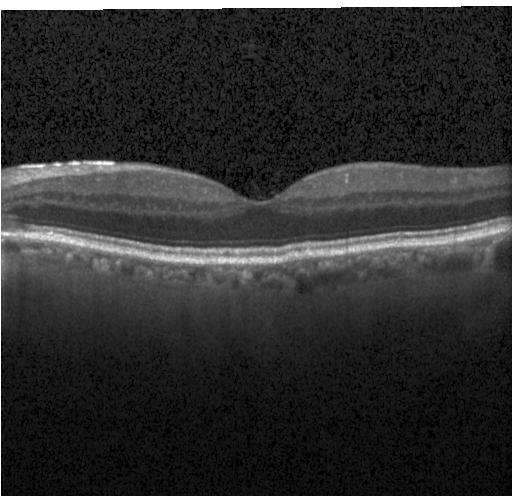

Retinal OCT B-scan. Impression: no evidence of choroidal neovascularization, diabetic macular edema, or drusen.